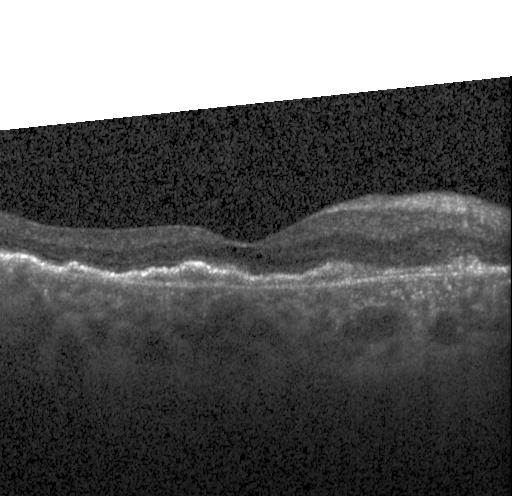

Heidelberg Spectralis · macular scan · spectral-domain optical coherence tomography · optical coherence tomography scan. OCT finding: a choroidal neovascular membrane.